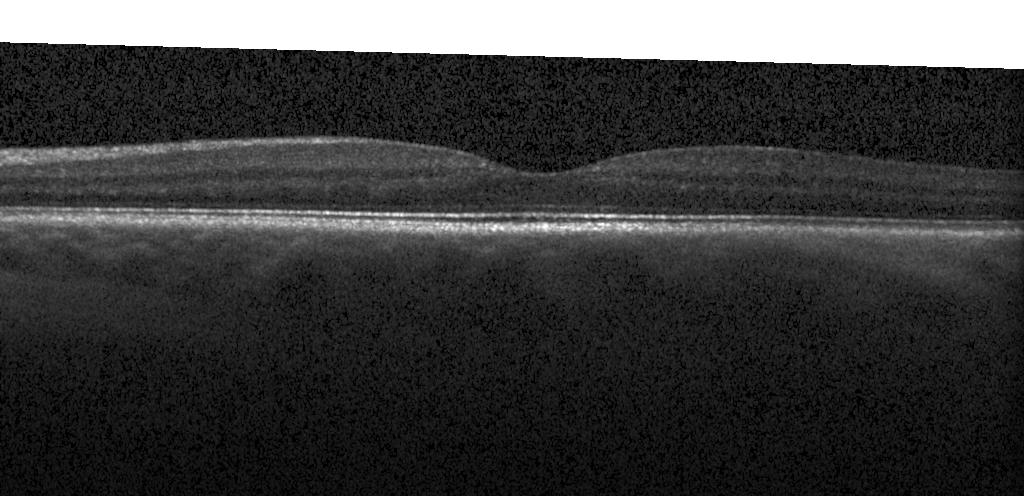
Retinal OCT B-scan
Diagnosis: no evidence of choroidal neovascularization, diabetic macular edema, or drusen.